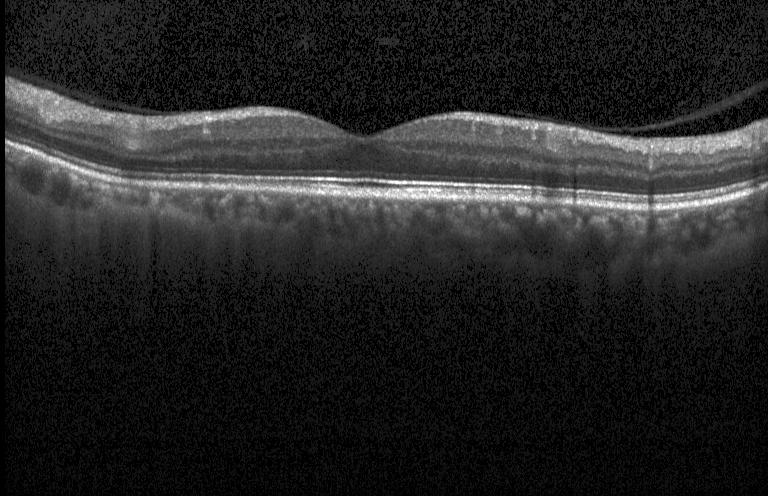
Instrument: Heidelberg Spectralis. Horizontal scan through the fovea. OCT line scan
The scan shows no evidence of CNV, DME, or drusen.